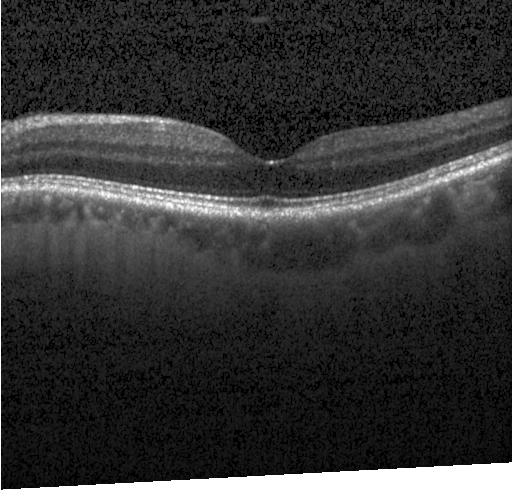

Centered on the fovea · OCT B-scan · Heidelberg Spectralis · SD-OCT — Finding: no evidence of choroidal neovascularization, diabetic macular edema, or drusen.